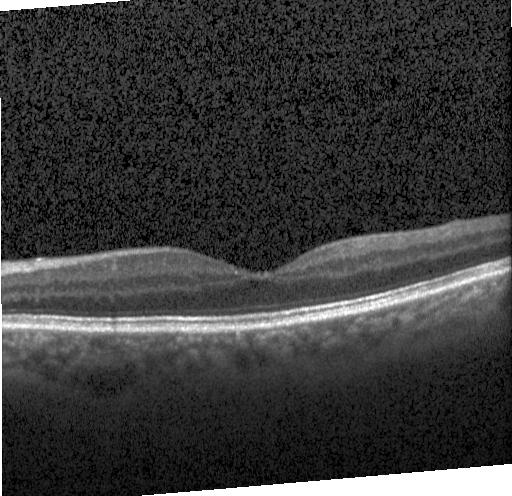
Instrument: Heidelberg Spectralis; optical coherence tomography scan — This B-scan demonstrates no choroidal neovascularization, diabetic macular edema, or drusen.